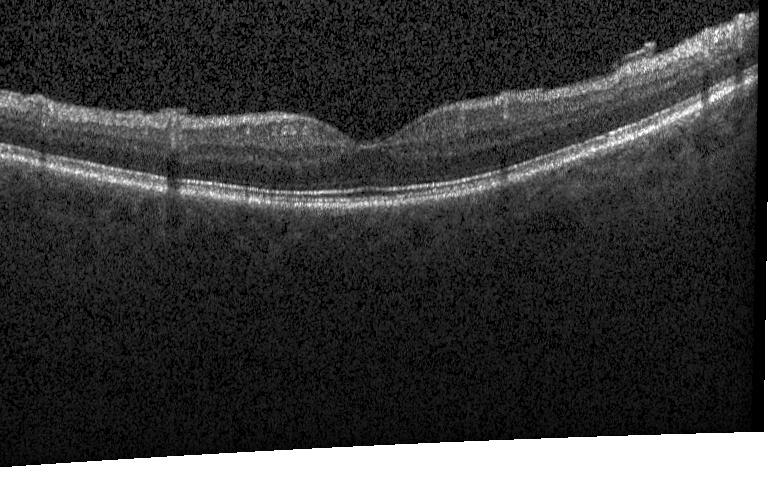
Optical coherence tomography scan, spectral-domain OCT
The scan shows no choroidal neovascularization, no diabetic macular edema, and no drusen.